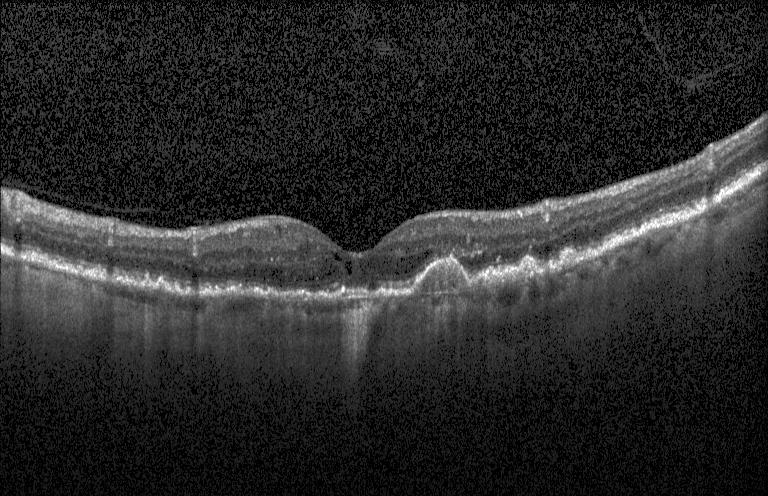
Retinal OCT B-scan
A choroidal neovascular membrane.